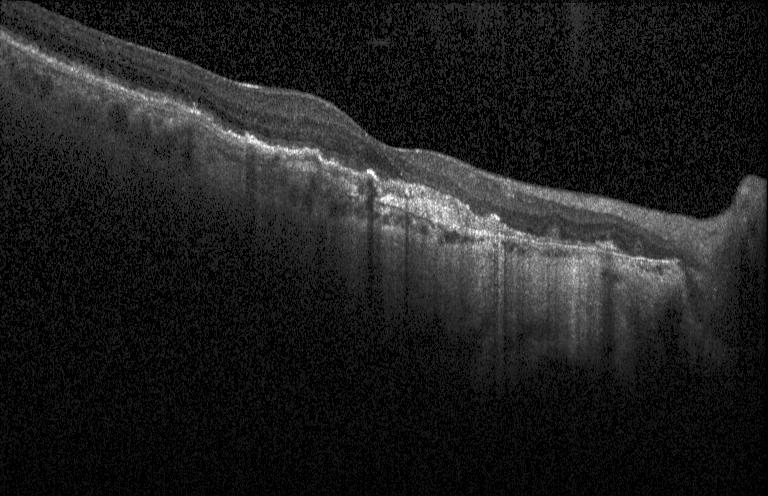 Impression: a choroidal neovascular membrane.